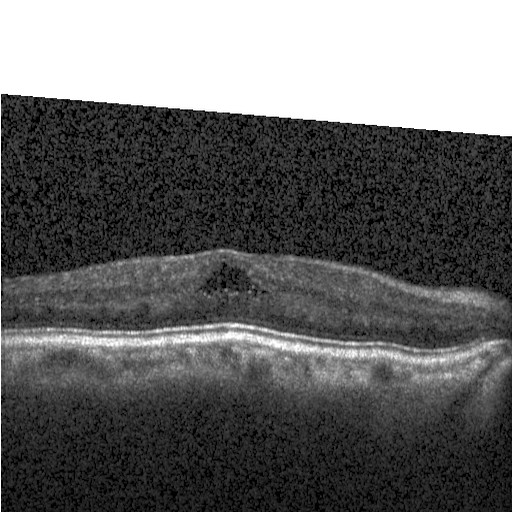

OCT B-scan — The scan shows diabetic macular edema (DME).